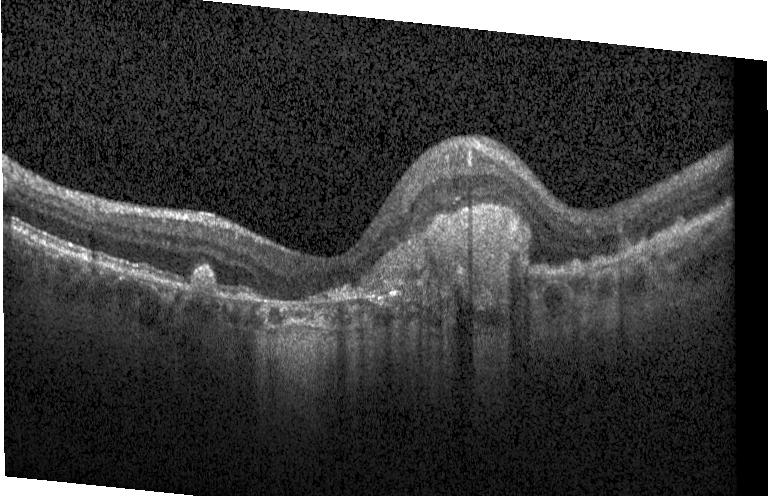

OCT finding: choroidal neovascularization (CNV).